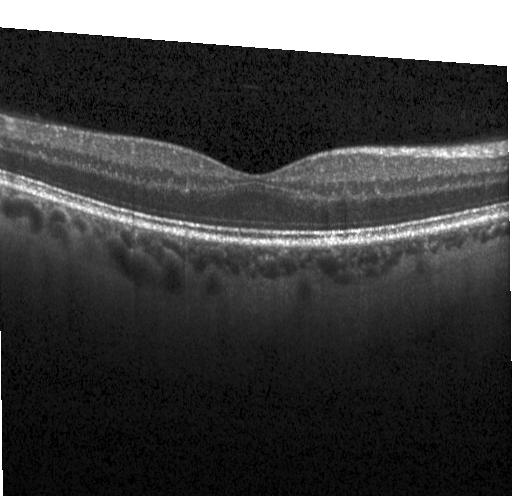
Optical coherence tomography B-scan · horizontal scan through the fovea. Impression: neither choroidal neovascularization, diabetic macular edema, nor drusen.